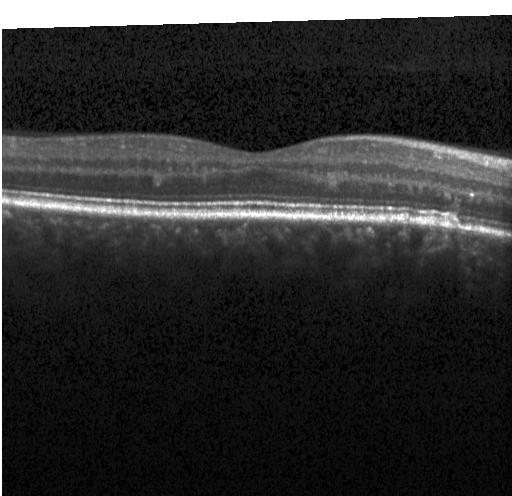
OCT line scan. This B-scan demonstrates no CNV, DME, or drusen.